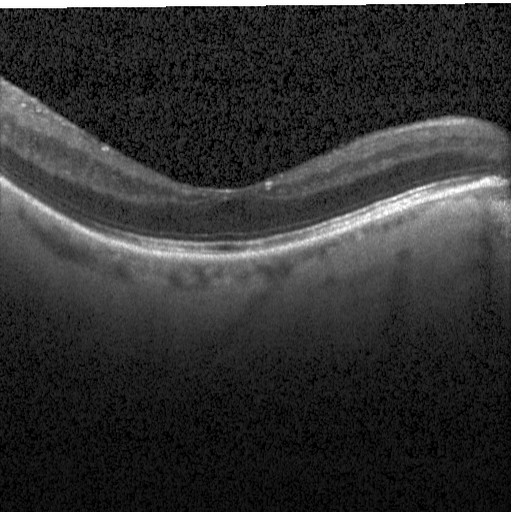
Spectral-domain optical coherence tomography, optical coherence tomography B-scan — Diabetic macular edema.